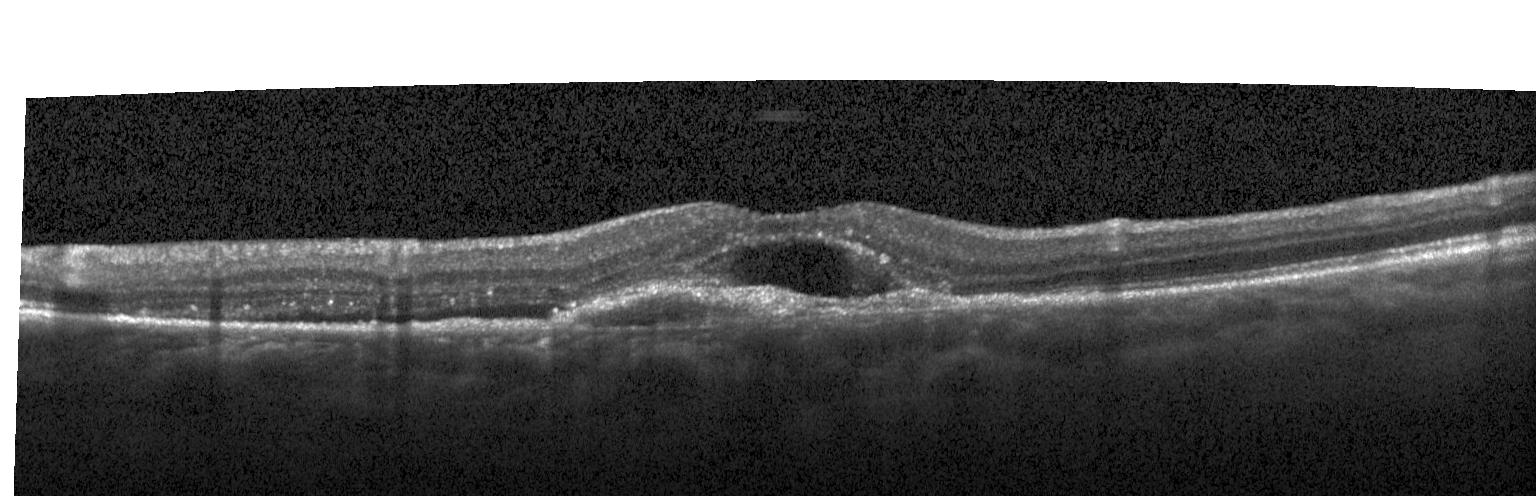
Assessment: a choroidal neovascular membrane.